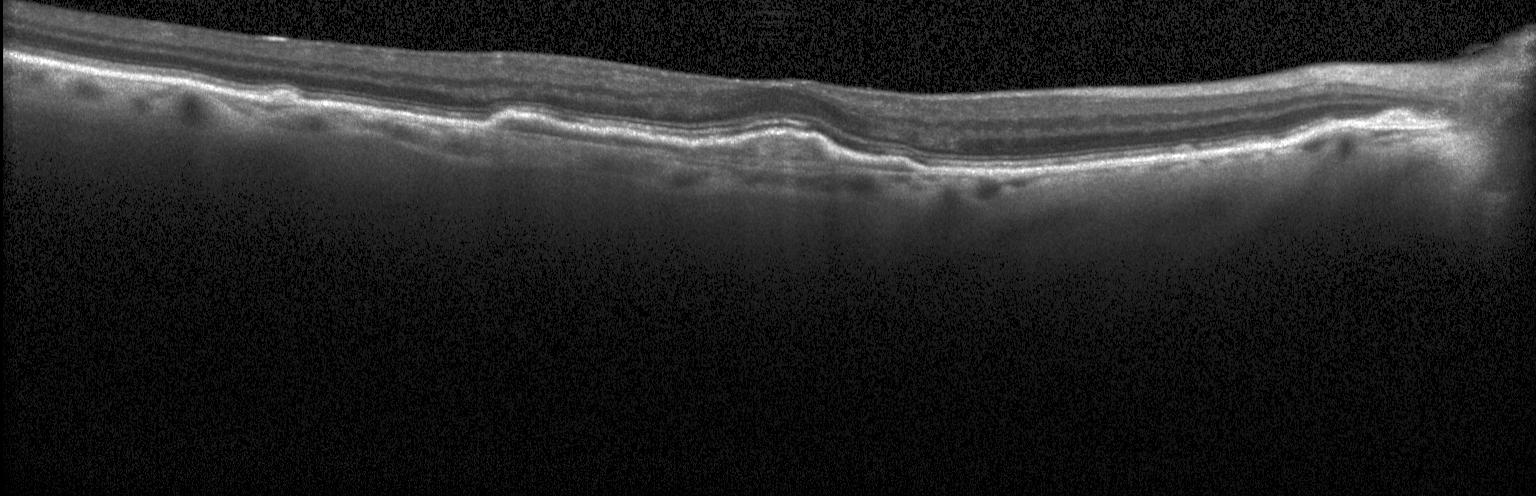
Diagnosis: choroidal neovascularization.